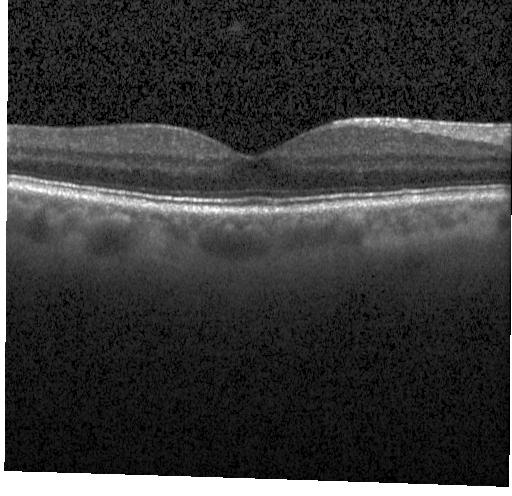 OCT B-scan, through the macula — This B-scan demonstrates neither CNV, DME, nor drusen.